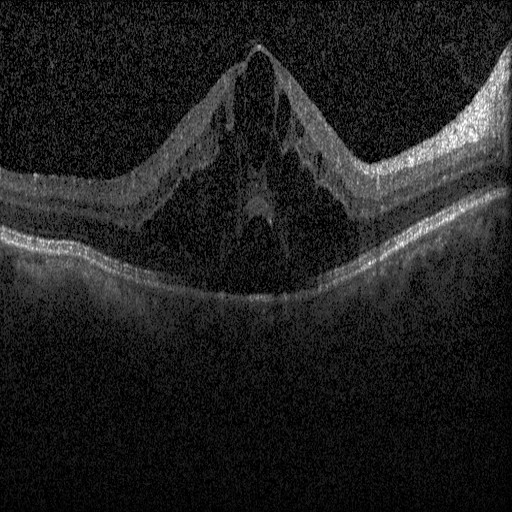 Centered on the fovea · OCT B-scan · spectral-domain optical coherence tomography · Heidelberg Spectralis OCT system
Diagnosis: diabetic macular edema.